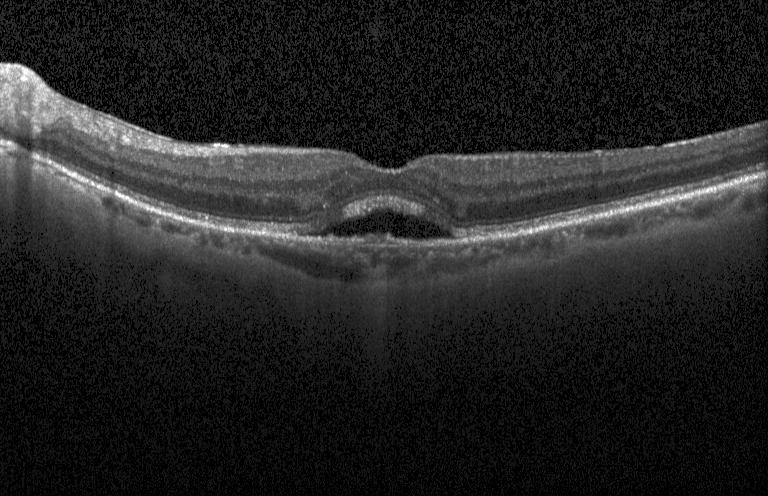
SD-OCT · retinal OCT B-scan · acquired on a Heidelberg Spectralis · horizontal scan through the fovea. Macular OCT: choroidal neovascularization.